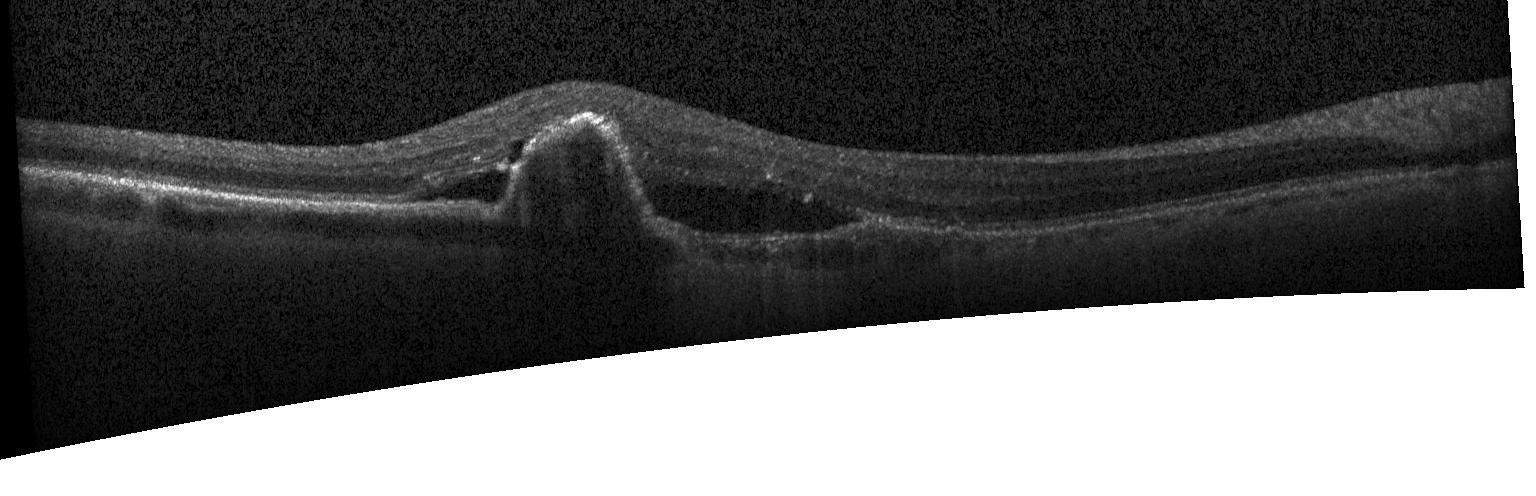

Spectral-domain optical coherence tomography · retinal OCT B-scan · horizontal scan through the fovea
Diagnosis: a choroidal neovascular membrane.